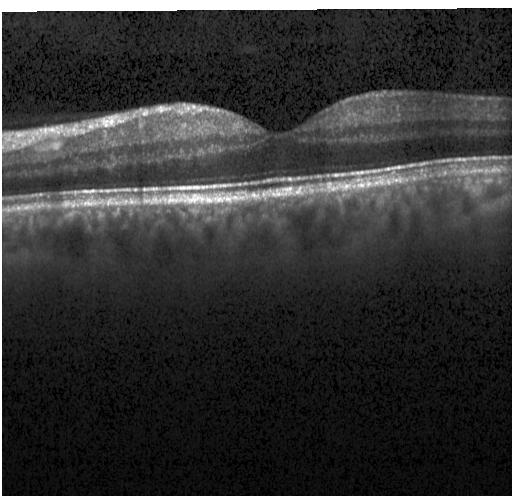 Centered on the fovea, SD-OCT, optical coherence tomography B-scan. Impression: no choroidal neovascularization, diabetic macular edema, or drusen.